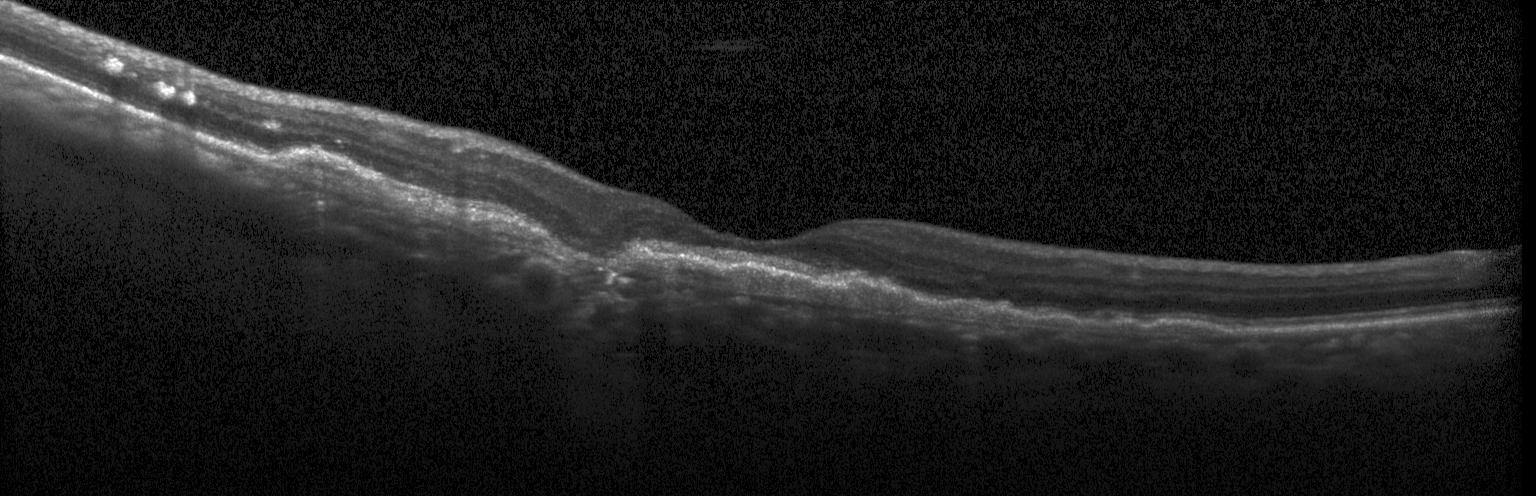
Spectral-domain OCT; OCT line scan; Heidelberg Spectralis OCT system. The scan shows a choroidal neovascular membrane.